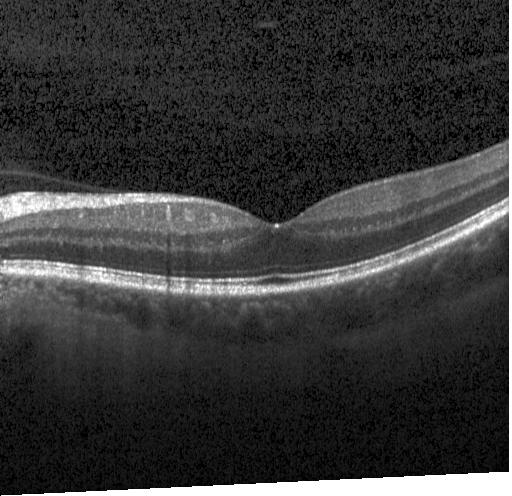
Macular OCT: no evidence of CNV, DME, or drusen.